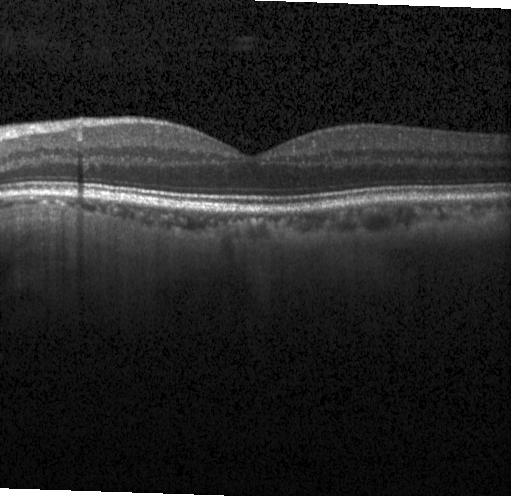

Fovea-centered, optical coherence tomography B-scan. Impression: no CNV, DME, or drusen.